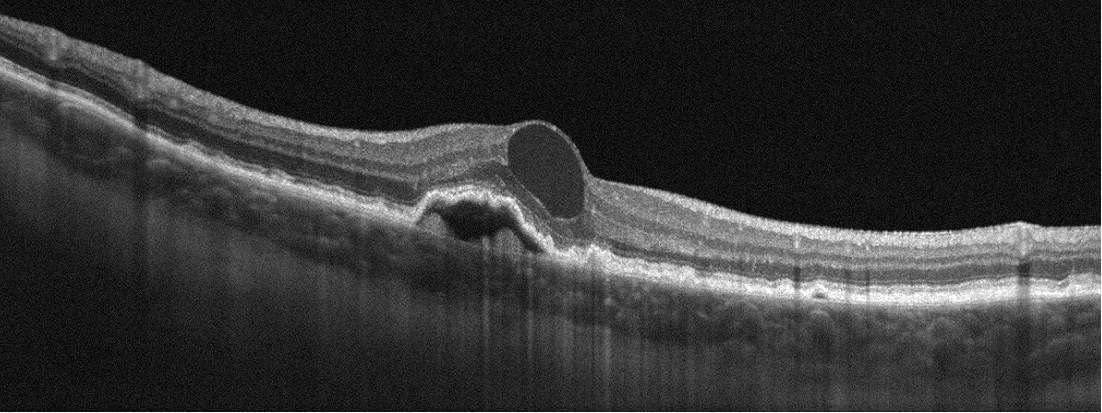
Fovea-centered · retinal OCT B-scan · Optovue Avanti RTVue XR — Assessment: AMD.